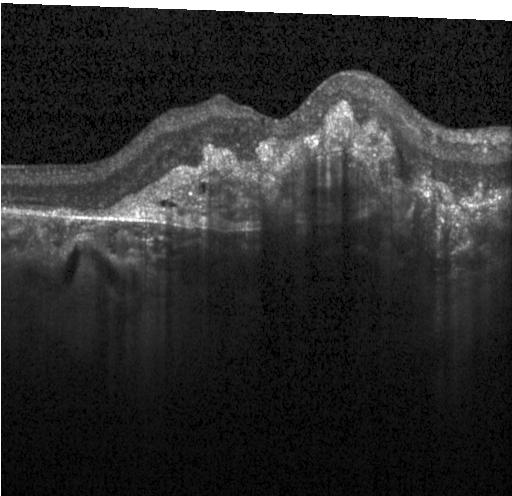

OCT B-scan; spectral-domain OCT — This B-scan demonstrates CNV.